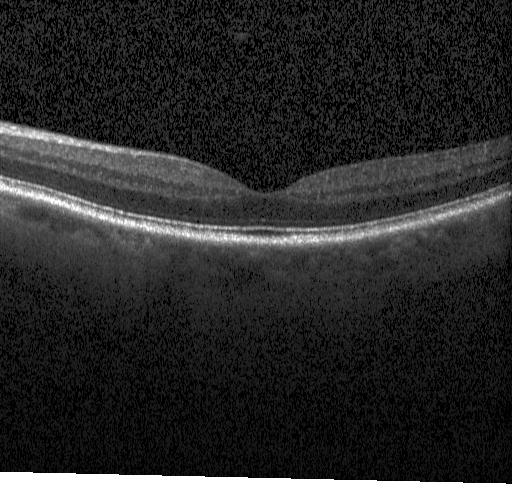
Retinal OCT B-scan. Macular scan. Impression: no evidence of choroidal neovascularization, diabetic macular edema, or drusen.